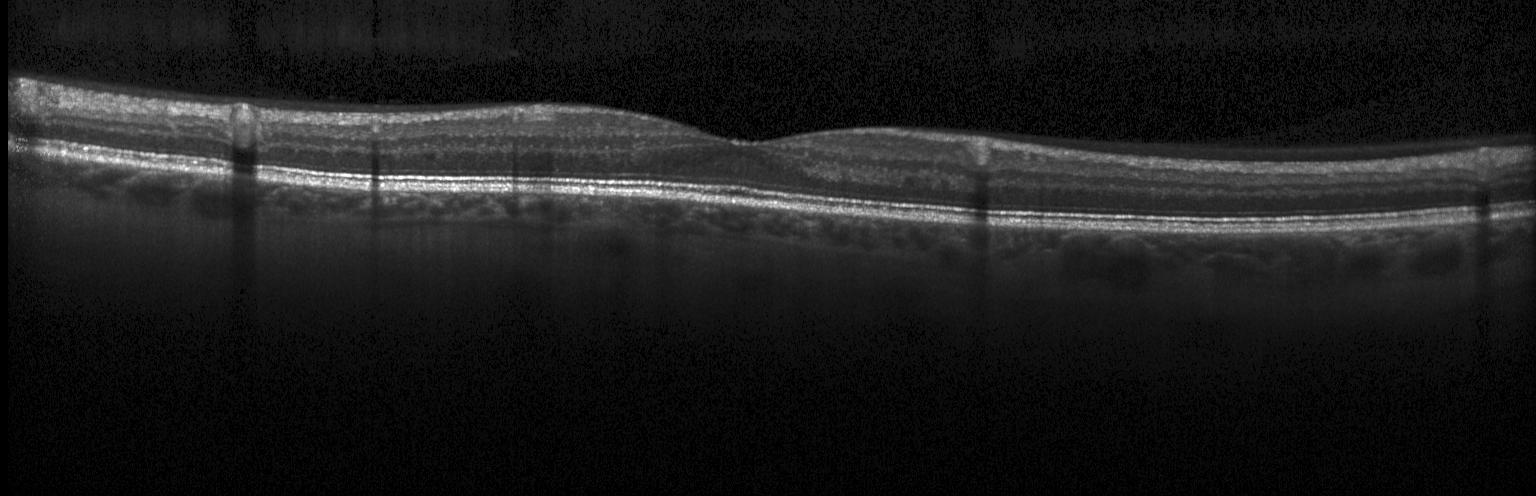
Finding: no choroidal neovascularization, no diabetic macular edema, and no drusen.